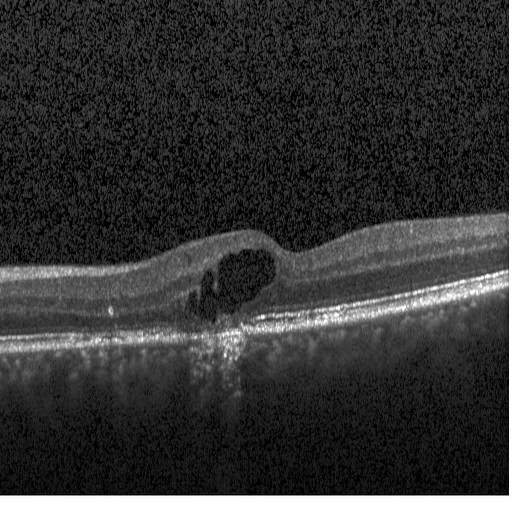

Retinal OCT B-scan; acquired on a Heidelberg Spectralis; SD-OCT. This B-scan demonstrates diabetic macular edema.